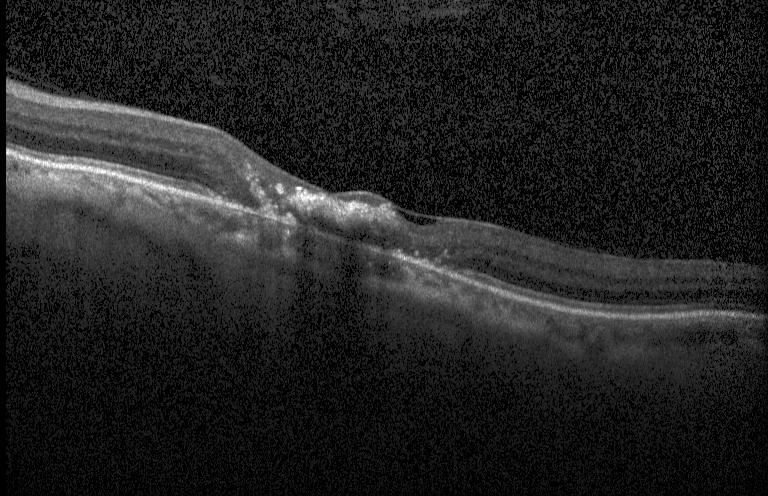
Acquired on a Heidelberg Spectralis. OCT B-scan. SD-OCT. Macular scan.
The scan shows a choroidal neovascular membrane.